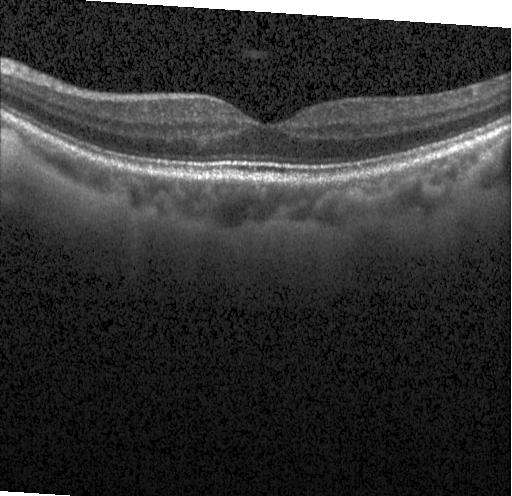 Heidelberg Spectralis OCT system · optical coherence tomography B-scan · SD-OCT. Finding: no choroidal neovascularization, no diabetic macular edema, and no drusen.